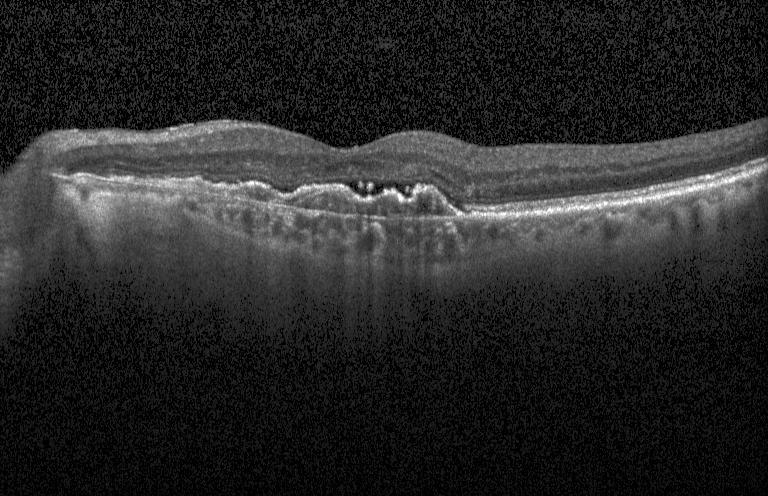 Spectral-domain optical coherence tomography; fovea-centered; Heidelberg Spectralis; optical coherence tomography scan.
Impression: choroidal neovascularization.